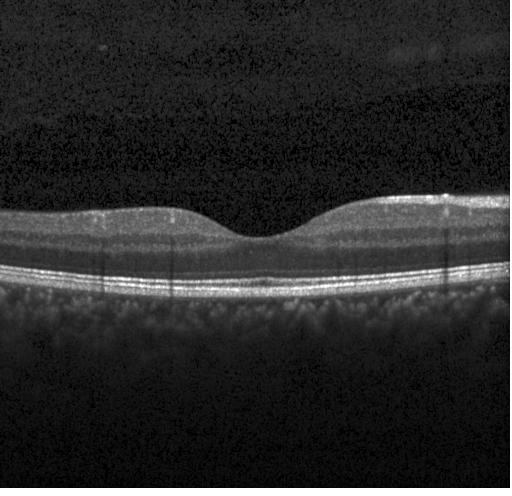
Spectral-domain OCT, optical coherence tomography B-scan, Heidelberg Spectralis, fovea-centered
Diagnosis: no choroidal neovascularization, no diabetic macular edema, and no drusen.